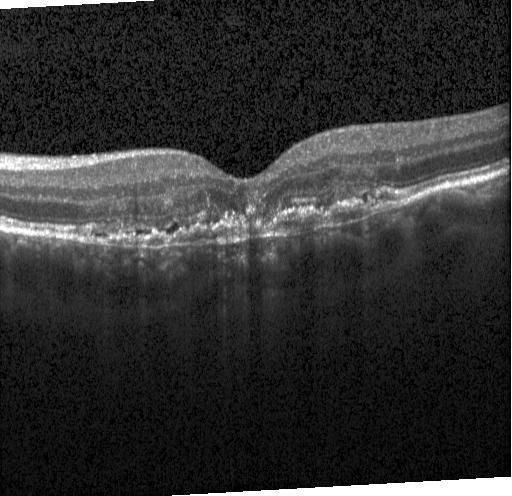
Macular OCT demonstrating a choroidal neovascular membrane.